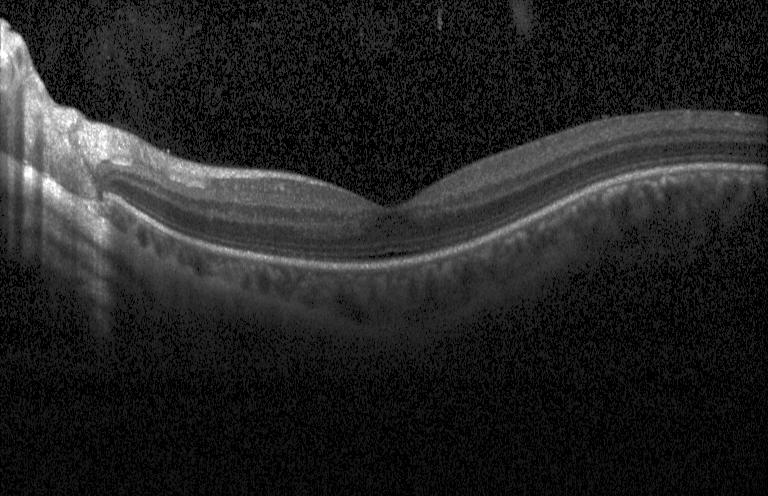

OCT finding: neither CNV, DME, nor drusen.